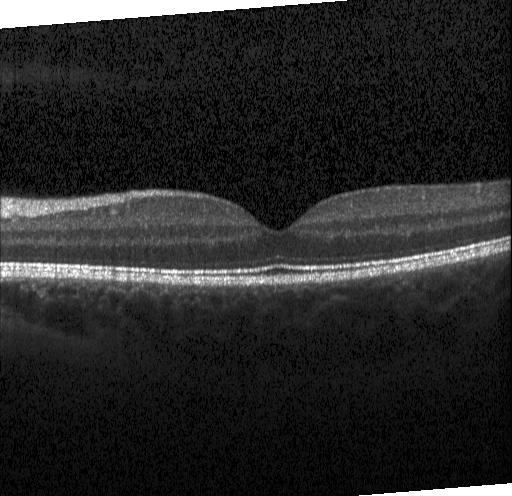 Optical coherence tomography B-scan · SD-OCT. Macular OCT: no evidence of choroidal neovascularization, diabetic macular edema, or drusen.